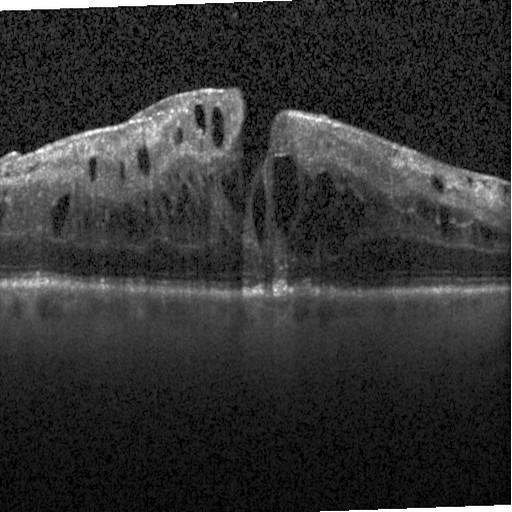

Through the macula. Optical coherence tomography scan. Heidelberg Spectralis. SD-OCT. Diagnosis: DME.